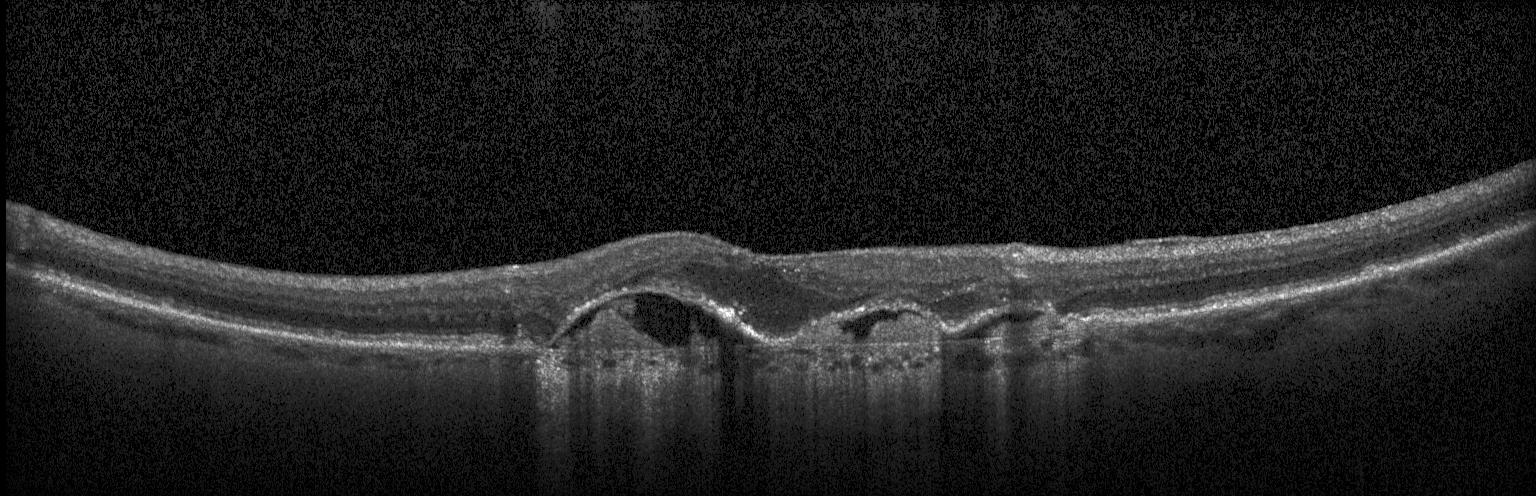
Retinal OCT B-scan. Diagnosis: a choroidal neovascular membrane.